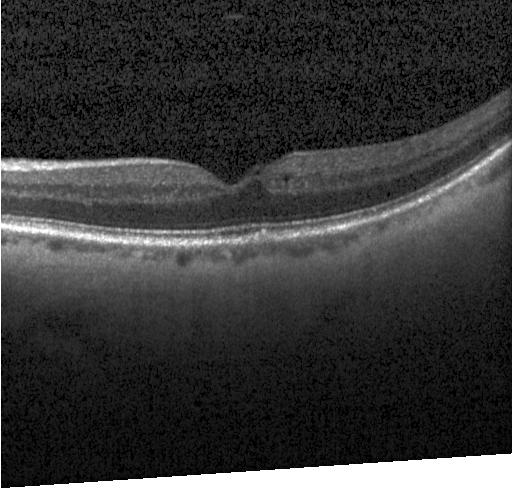
Horizontal scan through the fovea. Heidelberg Spectralis OCT system. Optical coherence tomography B-scan.
Diagnosis: diabetic macular edema.